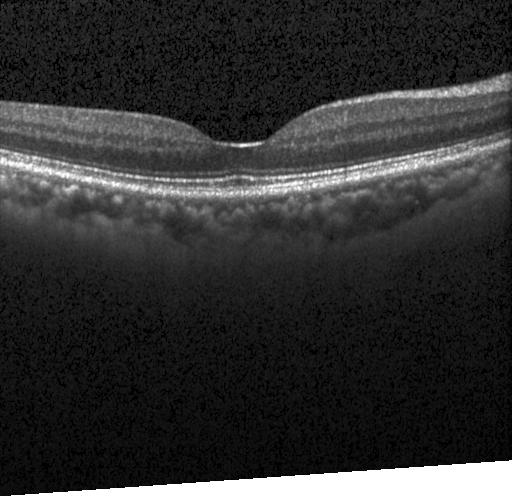
Spectral-domain OCT; retinal OCT cross-section; Heidelberg Spectralis; centered on the fovea. No evidence of choroidal neovascularization, diabetic macular edema, or drusen.